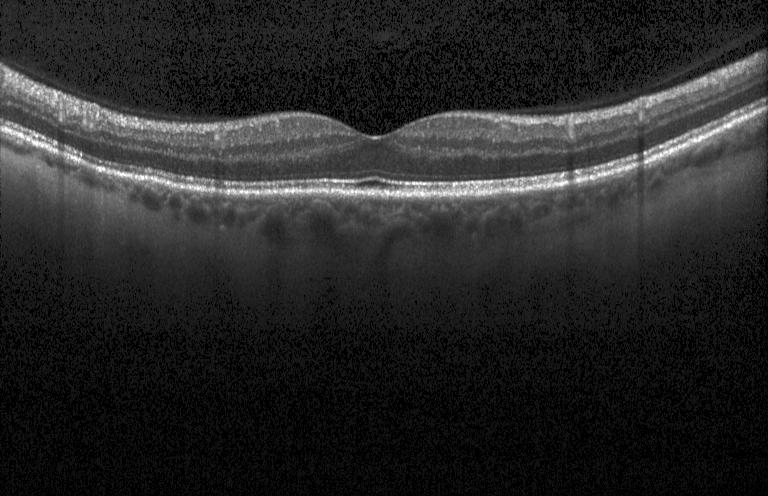

OCT line scan
Diagnosis: no evidence of CNV, DME, or drusen.